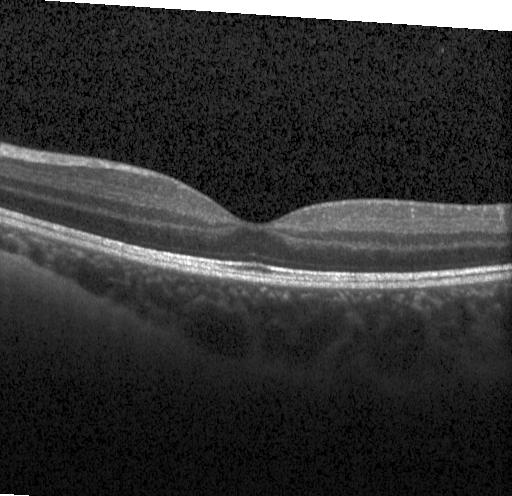
OCT scan showing no choroidal neovascularization, diabetic macular edema, or drusen.